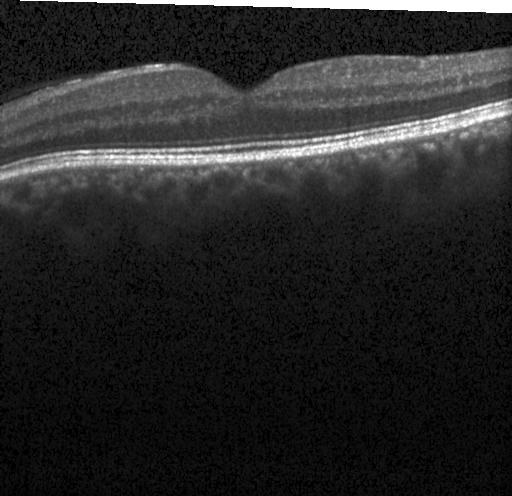 Retinal OCT B-scan. Diagnosis: no choroidal neovascularization, no diabetic macular edema, and no drusen.